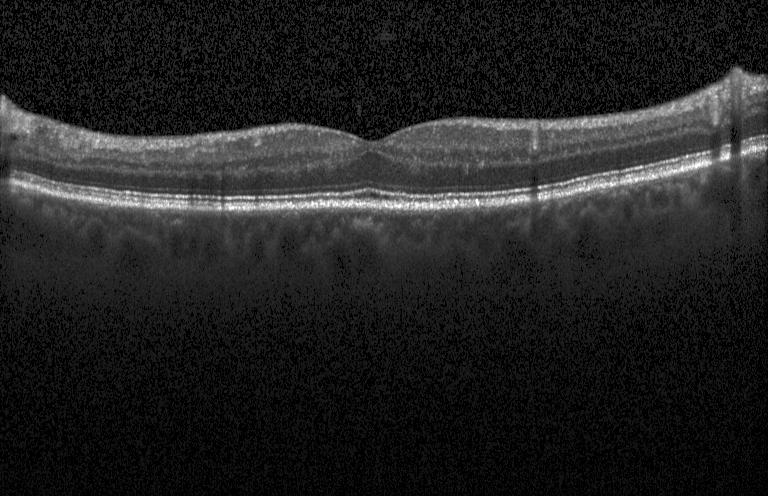
Retinal OCT cross-section, Heidelberg Spectralis, SD-OCT
Dx: no choroidal neovascularization, no diabetic macular edema, and no drusen.